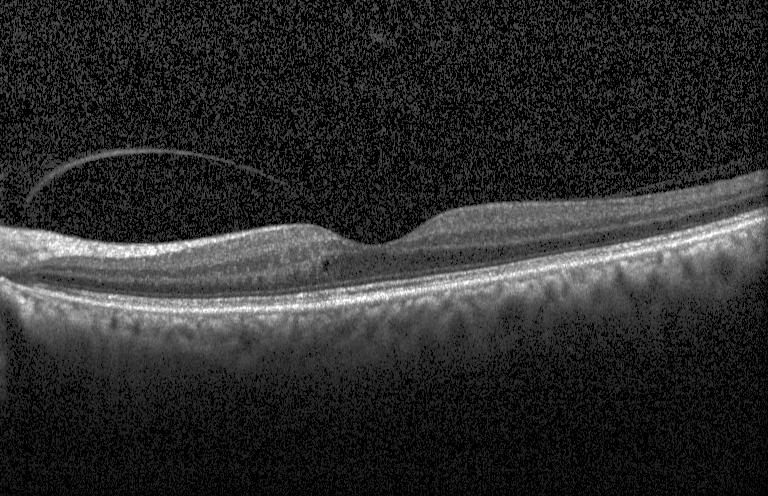 Finding: no evidence of CNV, DME, or drusen.